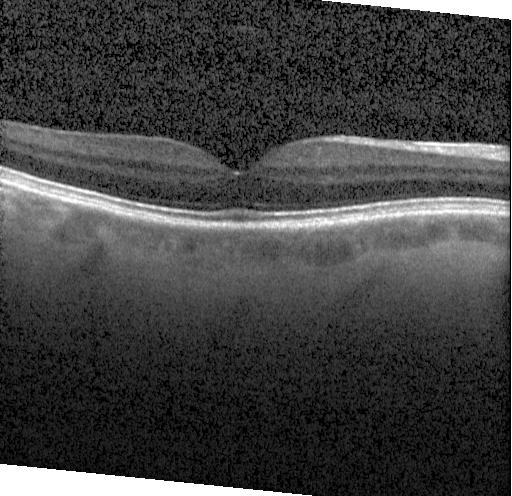

Assessment: no CNV, DME, or drusen.